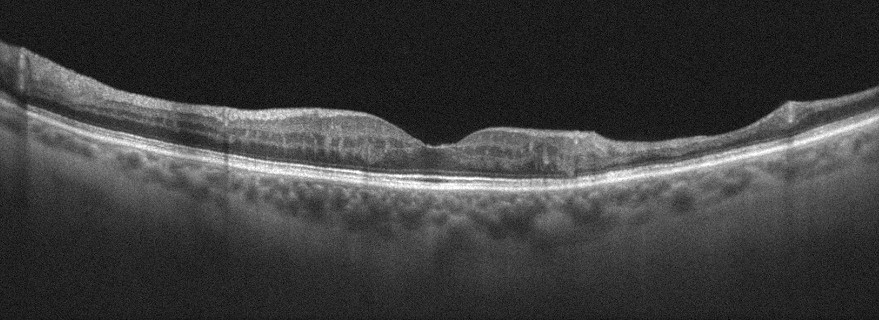
OCT line scan
Impression: retinal vein occlusion.